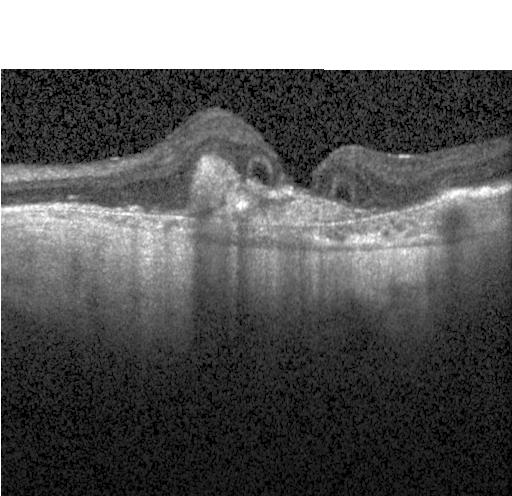
OCT B-scan.
Dx: a choroidal neovascular membrane.